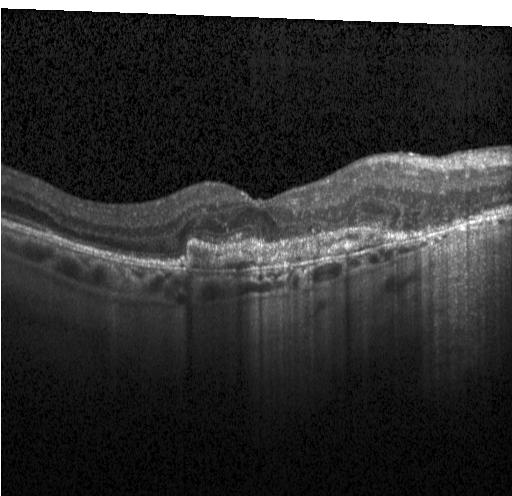

Spectral-domain optical coherence tomography · Heidelberg Spectralis · OCT B-scan — The scan shows a choroidal neovascular membrane.